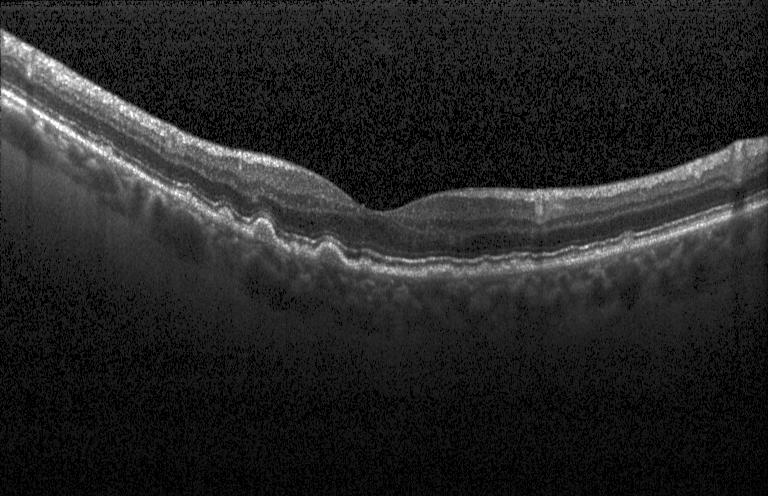 SD-OCT · OCT B-scan · horizontal scan through the fovea · acquired on a Heidelberg Spectralis — Diagnosis: drusen.